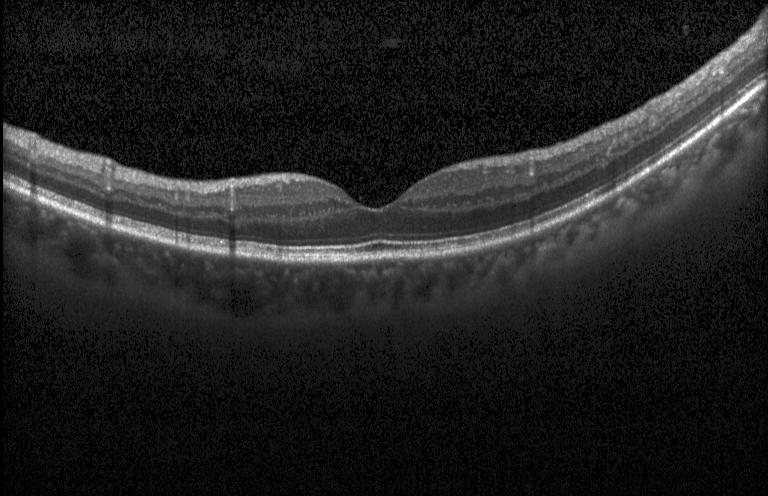

Finding: no CNV, DME, or drusen.